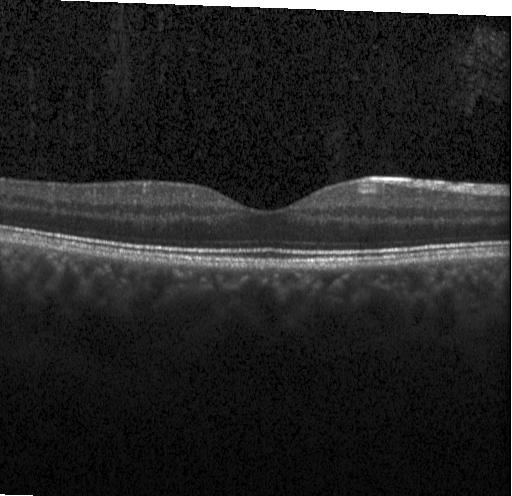
Retinal OCT cross-section showing no choroidal neovascularization, no diabetic macular edema, and no drusen.